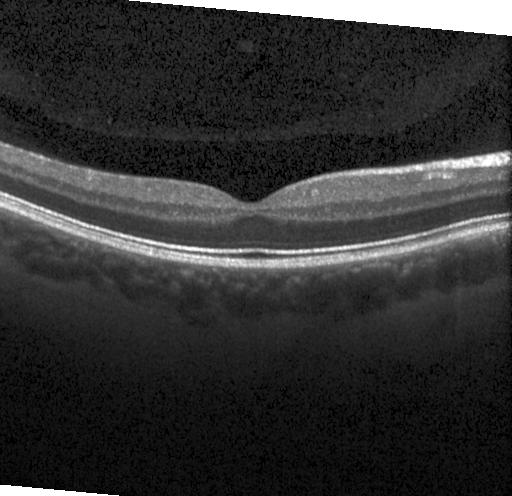

Assessment: no CNV, no DME, and no drusen.